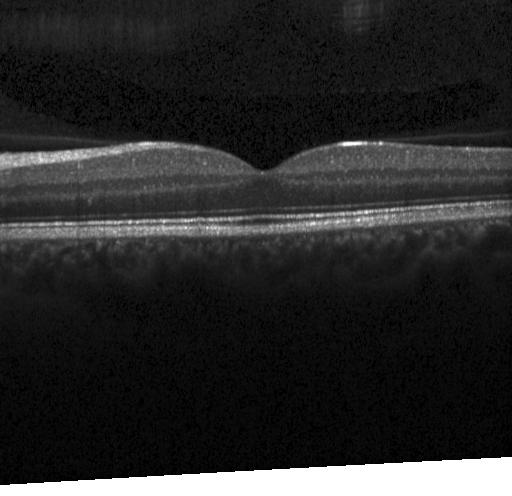 Heidelberg Spectralis OCT system, centered on the fovea, OCT line scan, spectral-domain optical coherence tomography — Diagnosis: no choroidal neovascularization, no diabetic macular edema, and no drusen.